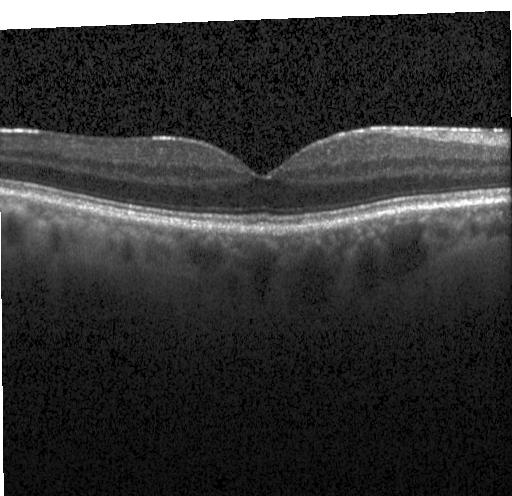

Spectral-domain optical coherence tomography · instrument: Heidelberg Spectralis · OCT B-scan · through the macula. OCT finding: no choroidal neovascularization, no diabetic macular edema, and no drusen.